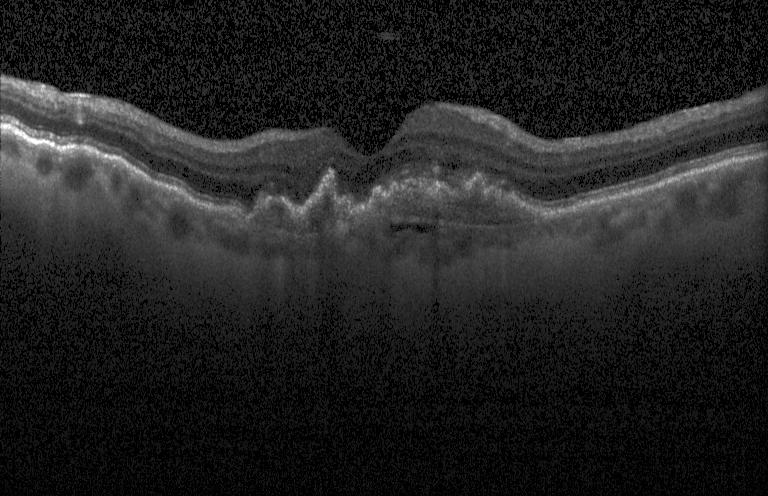

Retinal OCT cross-section; SD-OCT. Diagnosis: a choroidal neovascular membrane.